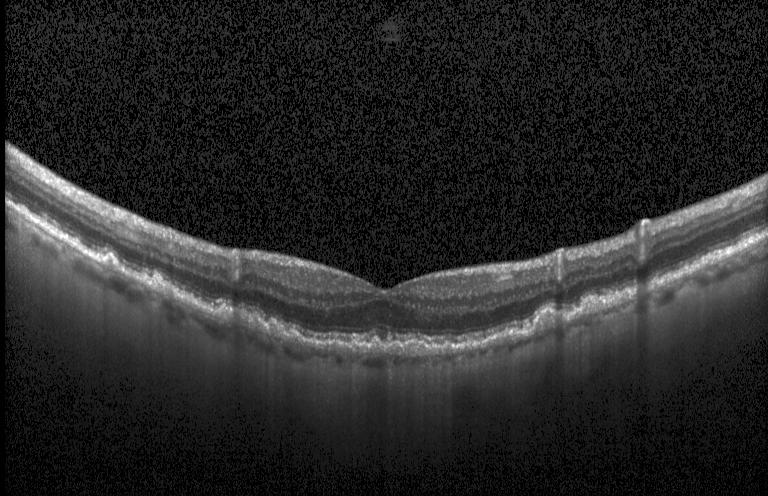 Optical coherence tomography scan. This B-scan demonstrates sub-RPE drusenoid deposits.